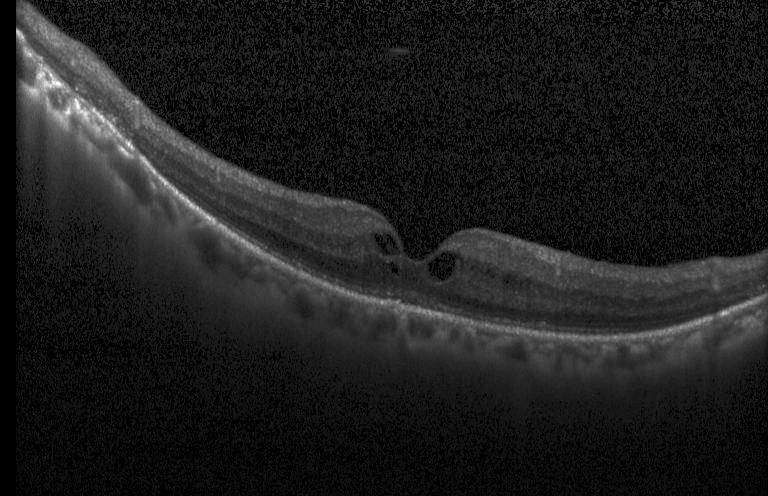

Heidelberg Spectralis; spectral-domain OCT; horizontal scan through the fovea; retinal OCT cross-section — Finding: diabetic macular edema (DME).